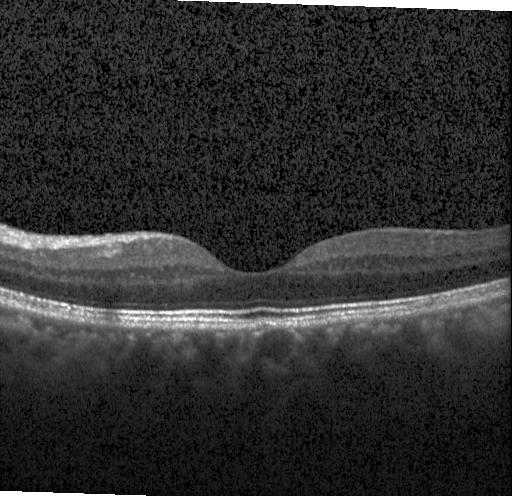 Spectral-domain optical coherence tomography · OCT line scan. Diagnosis: no evidence of choroidal neovascularization, diabetic macular edema, or drusen.